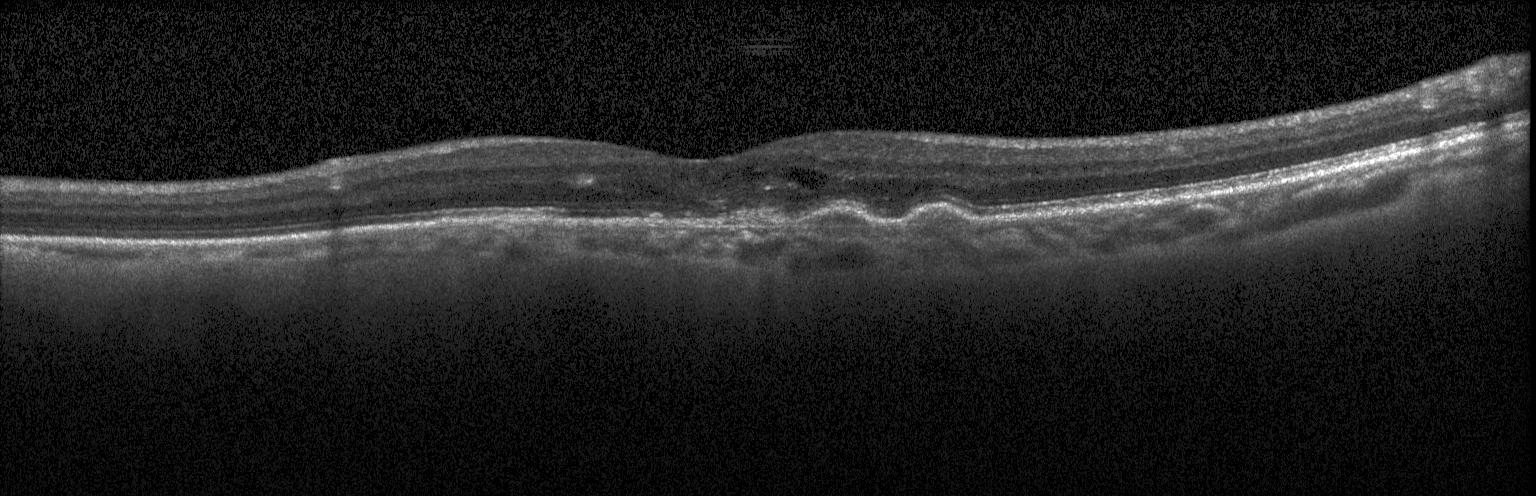 Optical coherence tomography scan; Heidelberg Spectralis OCT system; SD-OCT; macular scan.
A choroidal neovascular membrane.